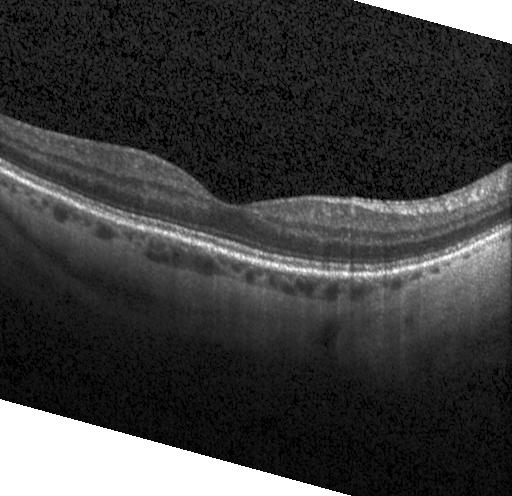
Diagnosis: no evidence of CNV, DME, or drusen.